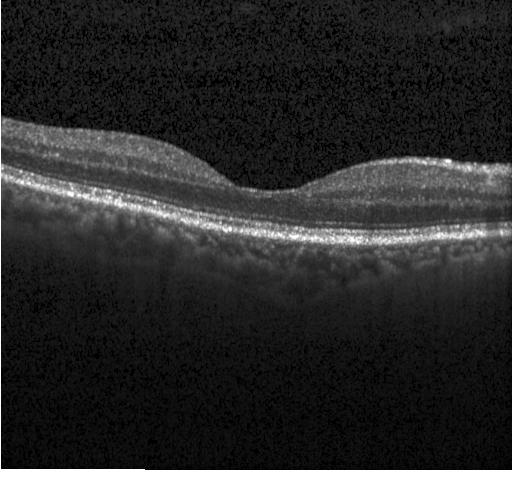

OCT B-scan. Spectral-domain OCT. OCT finding: no choroidal neovascularization, diabetic macular edema, or drusen.